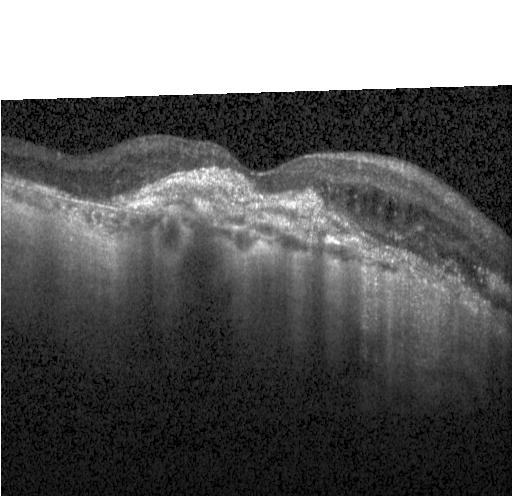

Spectral-domain optical coherence tomography, retinal OCT B-scan, acquired on a Heidelberg Spectralis, fovea-centered.
Impression: CNV.